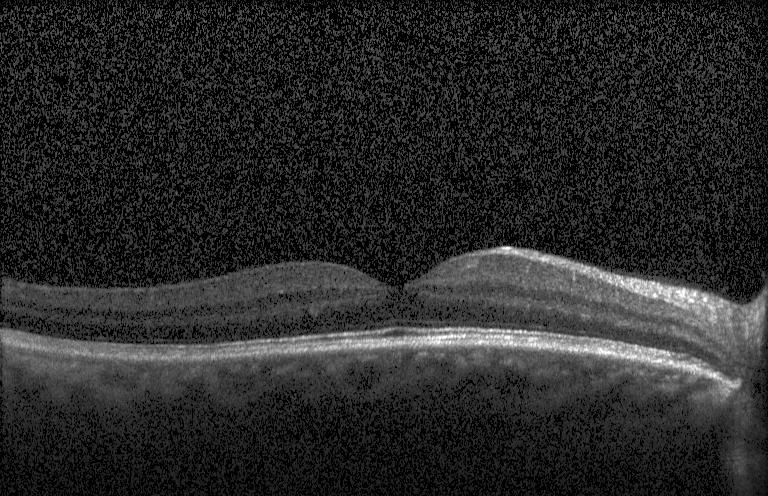 Dx: neither choroidal neovascularization, diabetic macular edema, nor drusen.